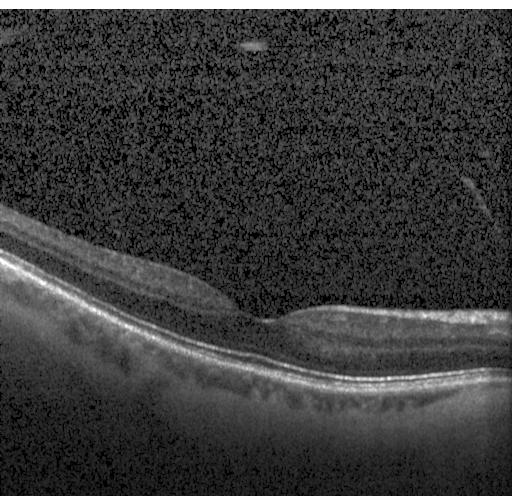 Optical coherence tomography B-scan — Diagnosis: no evidence of choroidal neovascularization, diabetic macular edema, or drusen.